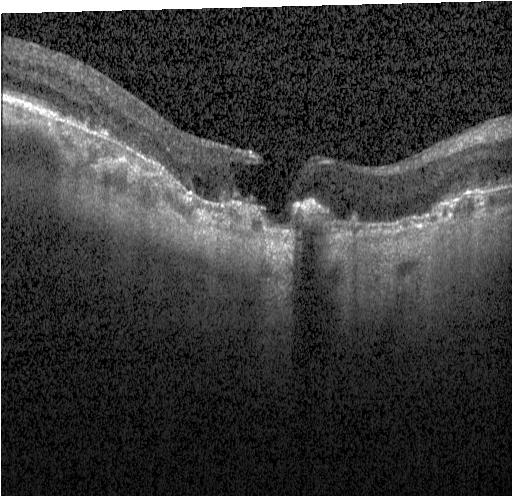
Optical coherence tomography scan; horizontal scan through the fovea; Heidelberg Spectralis. Assessment: a choroidal neovascular membrane.